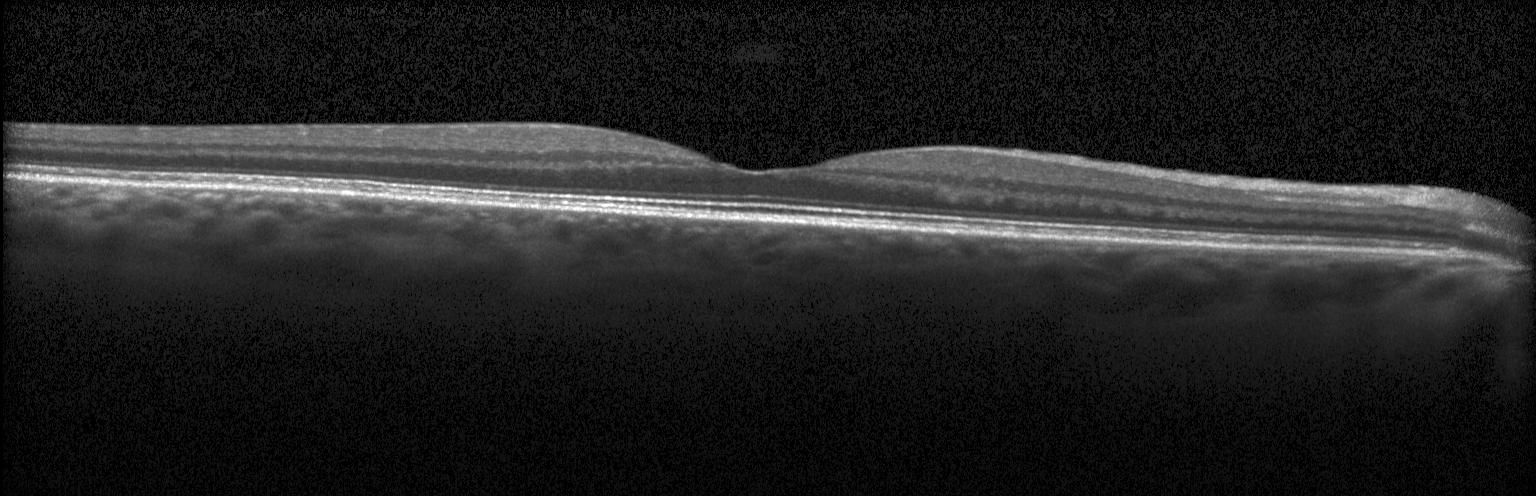
The scan shows no choroidal neovascularization, no diabetic macular edema, and no drusen.